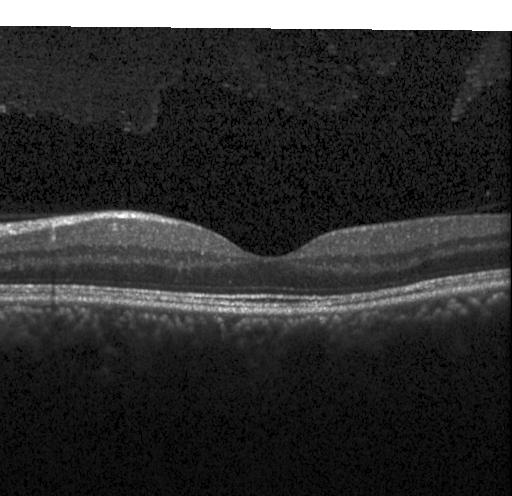 OCT B-scan. No CNV, DME, or drusen.